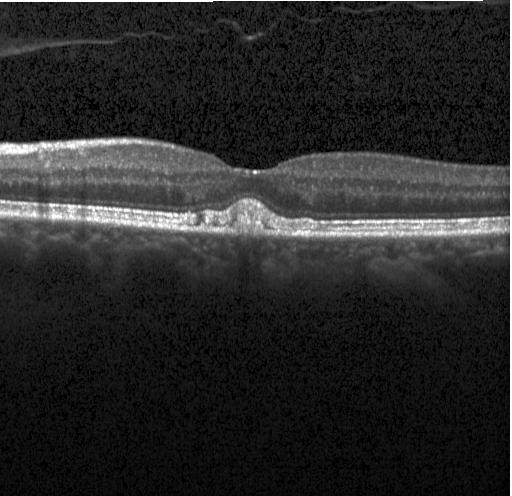

This B-scan demonstrates drusen.